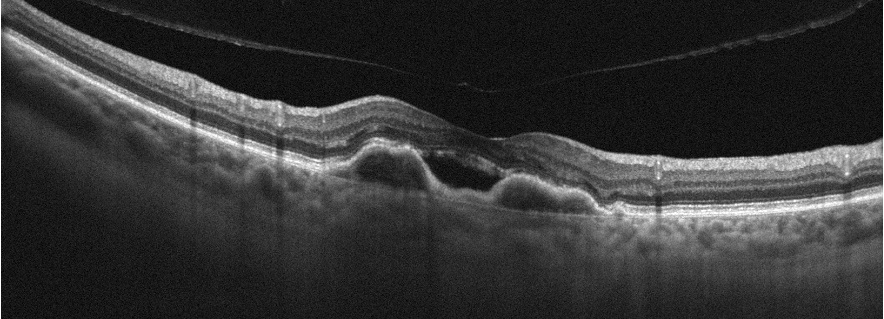 OCT B-scan showing age-related macular degeneration.